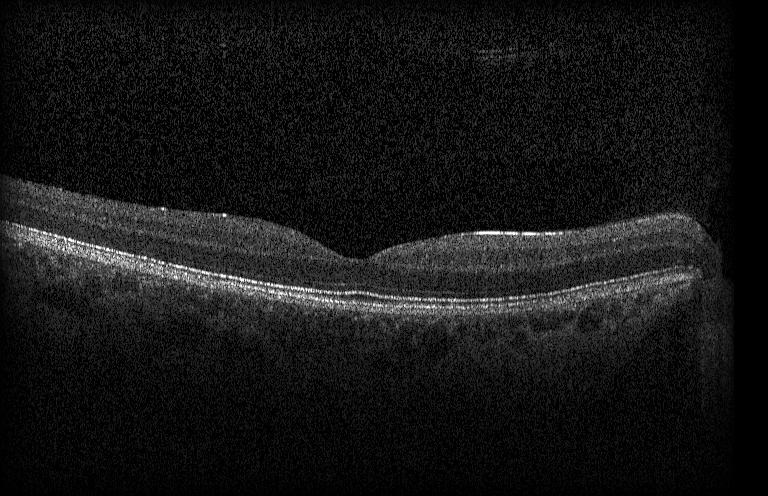
OCT line scan.
Finding: neither choroidal neovascularization, diabetic macular edema, nor drusen.